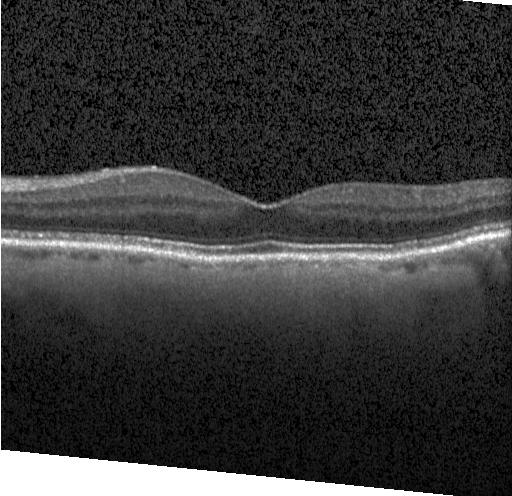

Spectral-domain OCT B-scan: neither choroidal neovascularization, diabetic macular edema, nor drusen.